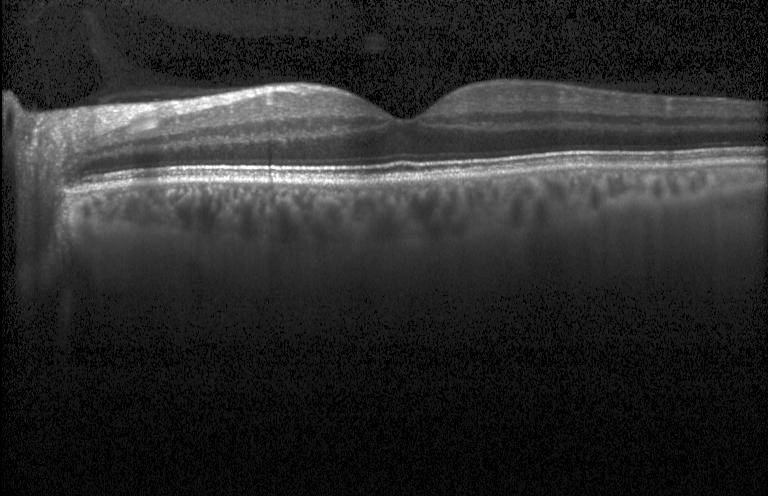 Instrument: Heidelberg Spectralis. Retinal OCT cross-section. Through the macula. Spectral-domain optical coherence tomography. Impression: neither choroidal neovascularization, diabetic macular edema, nor drusen.